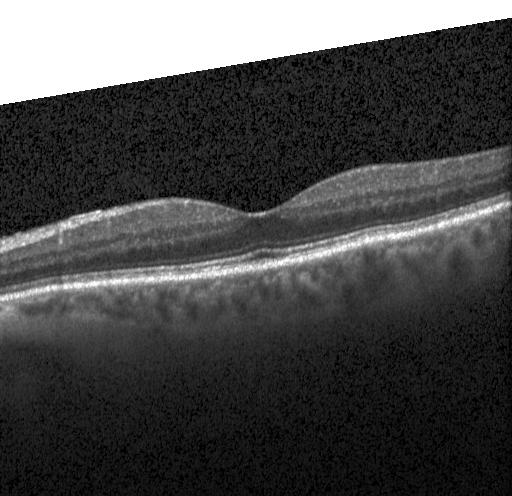
Heidelberg Spectralis OCT system · OCT B-scan · spectral-domain OCT
Macular OCT: no evidence of choroidal neovascularization, diabetic macular edema, or drusen.